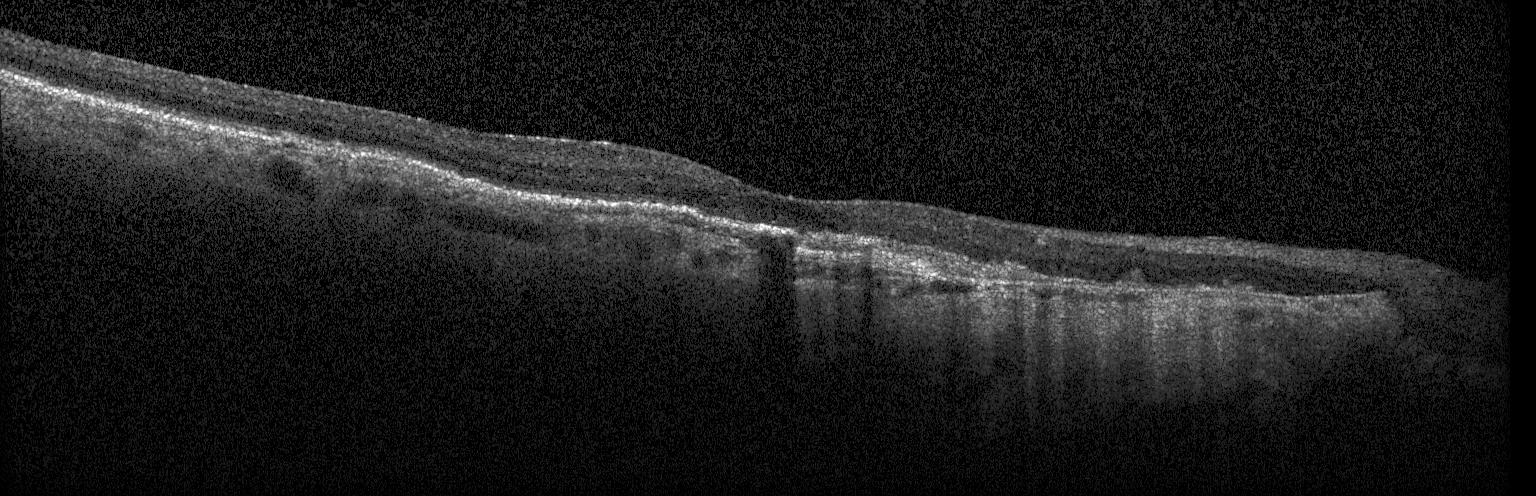

Horizontal scan through the fovea, Heidelberg Spectralis, OCT B-scan, spectral-domain optical coherence tomography. A choroidal neovascular membrane.